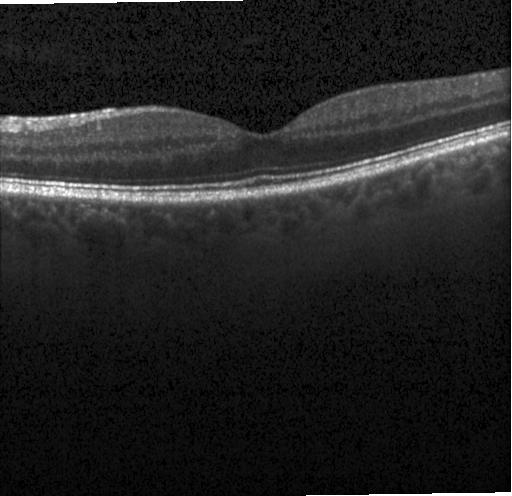

This B-scan demonstrates neither CNV, DME, nor drusen.